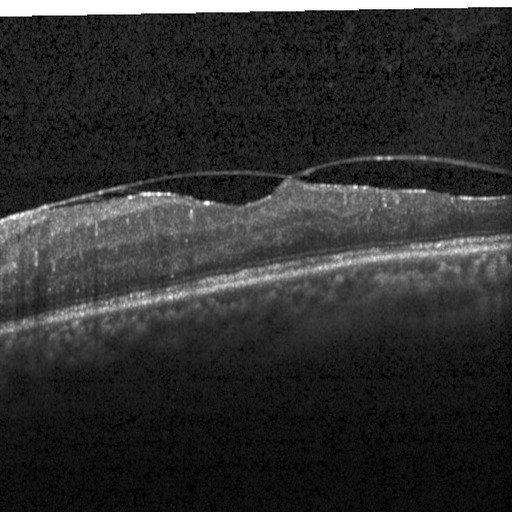 Dx: diabetic macular edema (DME).